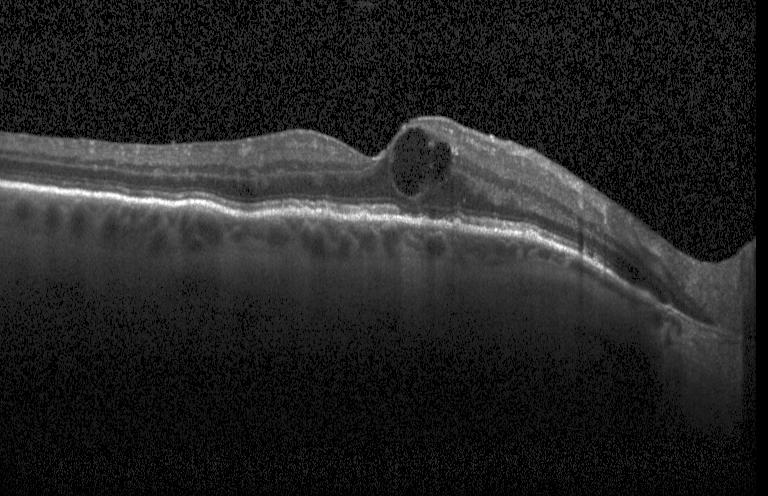

Fovea-centered · optical coherence tomography B-scan. Dx: a choroidal neovascular membrane.